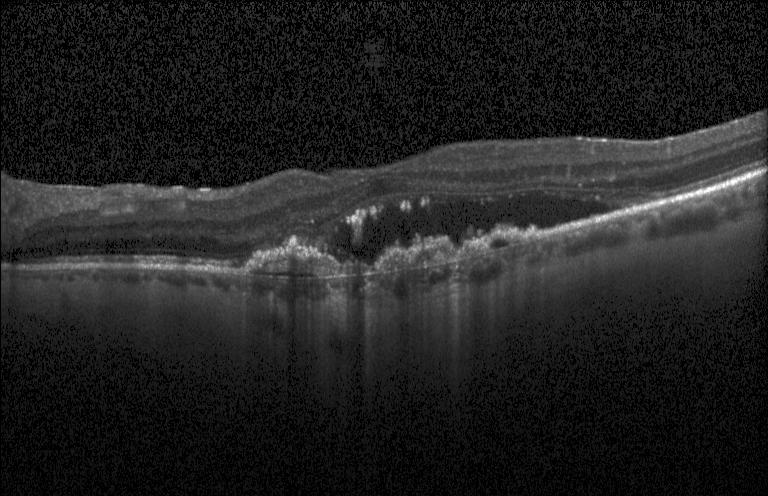

Retinal OCT B-scan · spectral-domain OCT · fovea-centered — This B-scan demonstrates a choroidal neovascular membrane.